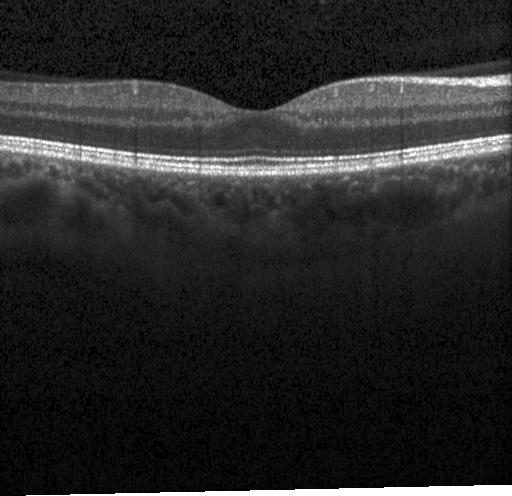 Macular OCT demonstrating no choroidal neovascularization, diabetic macular edema, or drusen.